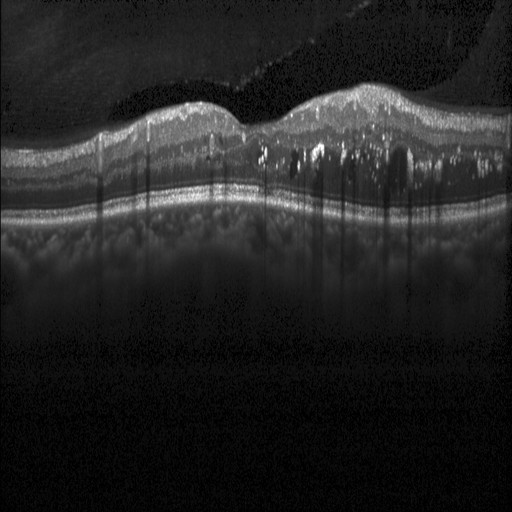
Horizontal scan through the fovea; retinal OCT cross-section; spectral-domain optical coherence tomography; Heidelberg Spectralis.
Assessment: diabetic macular edema (DME).